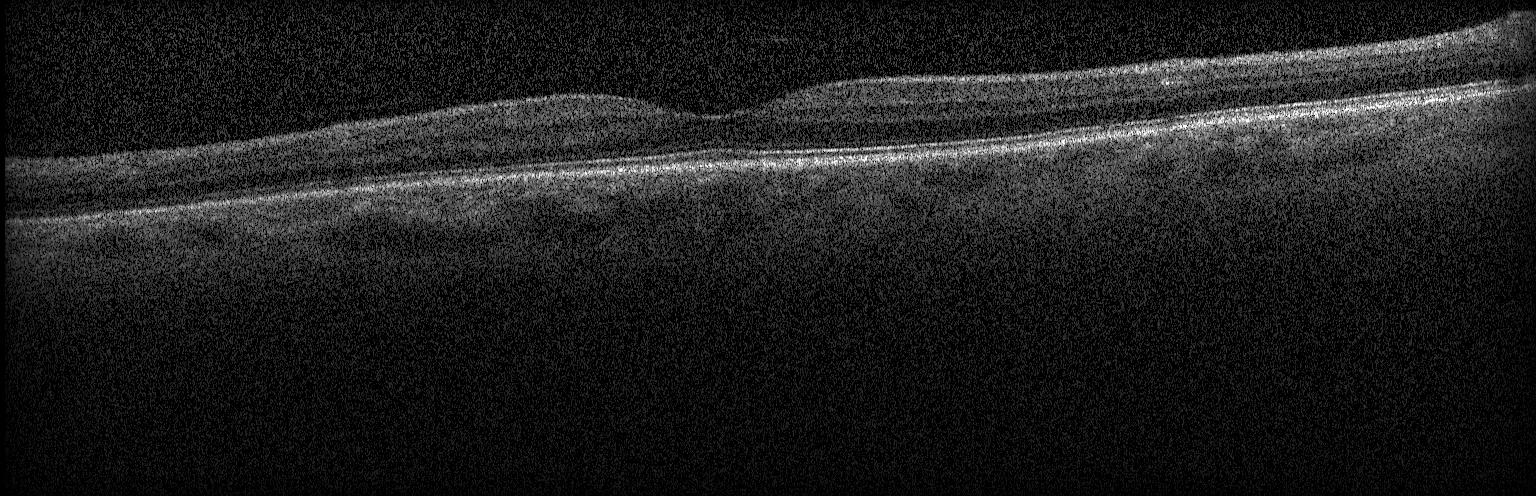
OCT B-scan. Fovea-centered. Spectral-domain OCT.
Diagnosis: neither choroidal neovascularization, diabetic macular edema, nor drusen.